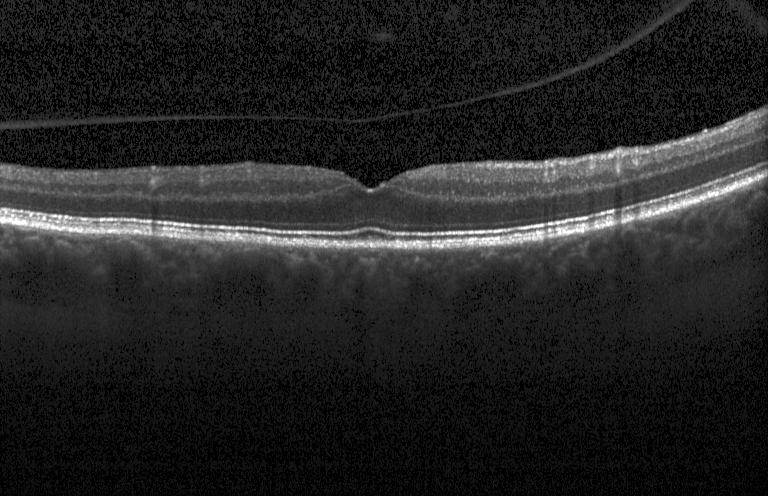
Retinal OCT B-scan; centered on the fovea. OCT finding: no evidence of CNV, DME, or drusen.